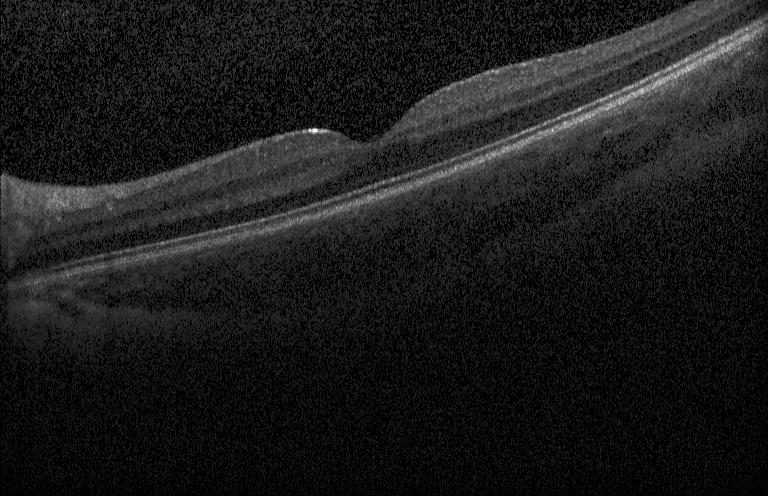
Optical coherence tomography scan, Heidelberg Spectralis OCT system.
The scan shows no choroidal neovascularization, diabetic macular edema, or drusen.